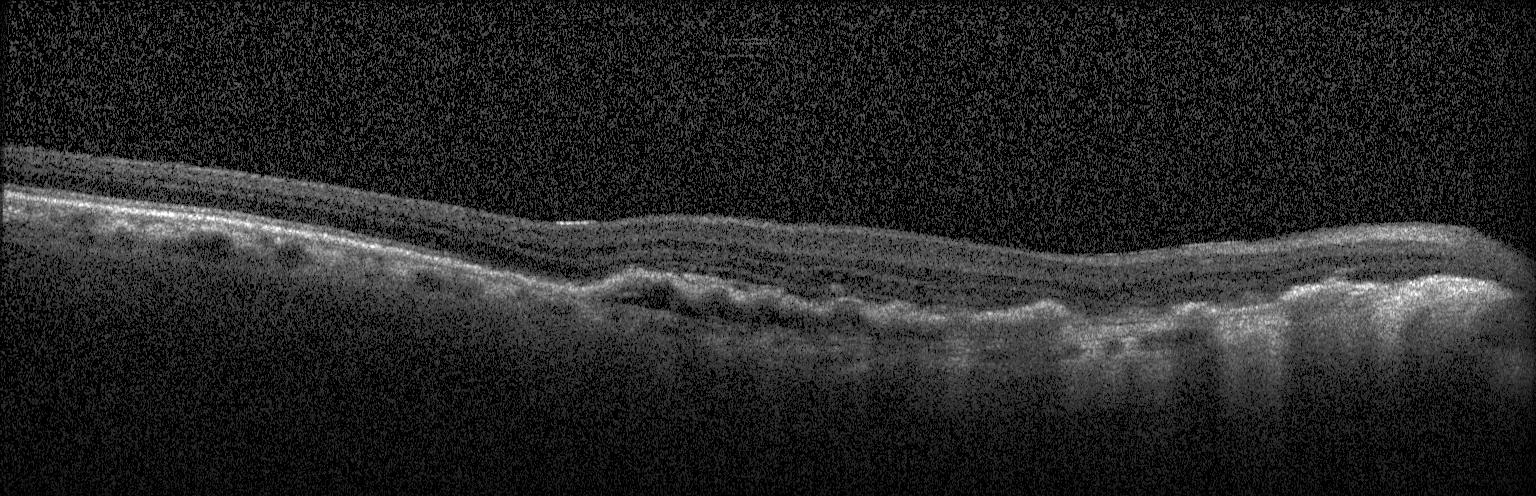 OCT line scan; spectral-domain optical coherence tomography; acquired on a Heidelberg Spectralis.
Impression: a choroidal neovascular membrane.